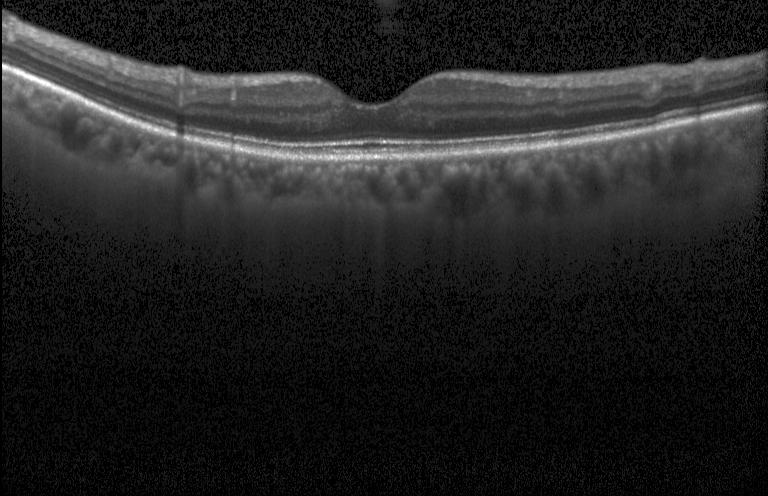

Spectral-domain OCT B-scan: no choroidal neovascularization, no diabetic macular edema, and no drusen.